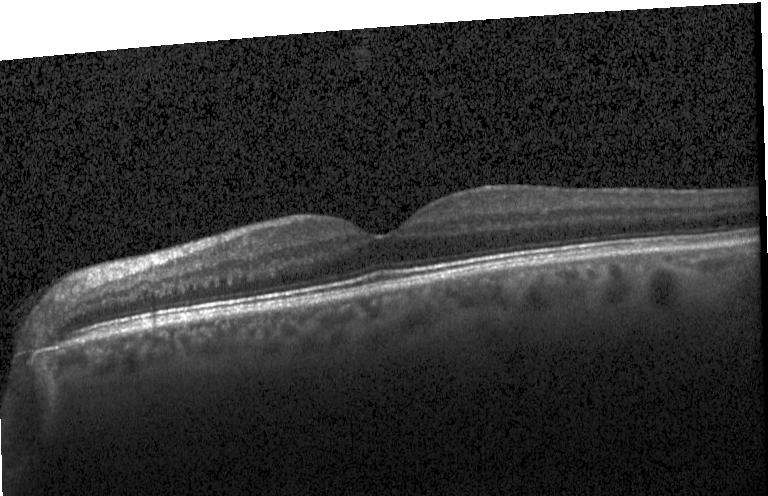

Retinal OCT B-scan.
Dx: no choroidal neovascularization, no diabetic macular edema, and no drusen.